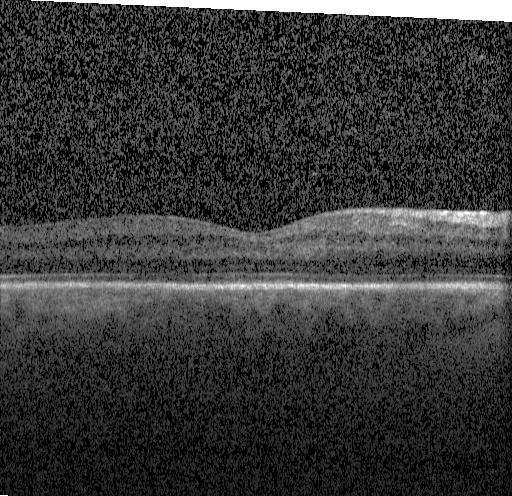

Macular OCT: no choroidal neovascularization, no diabetic macular edema, and no drusen.